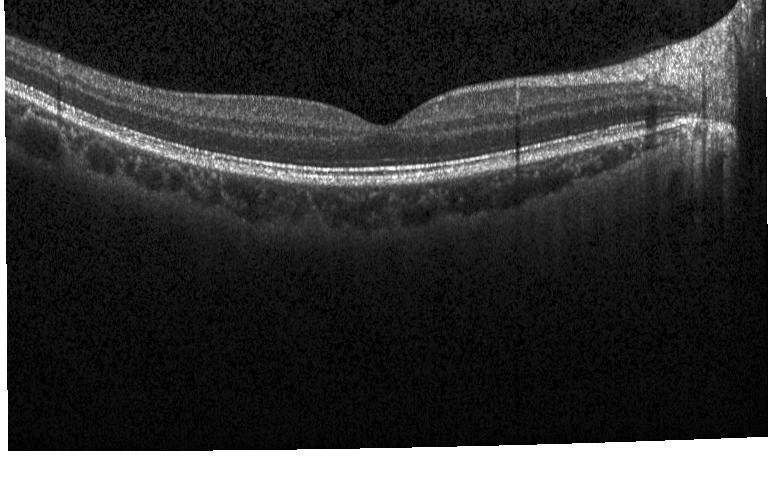
Assessment: neither choroidal neovascularization, diabetic macular edema, nor drusen.